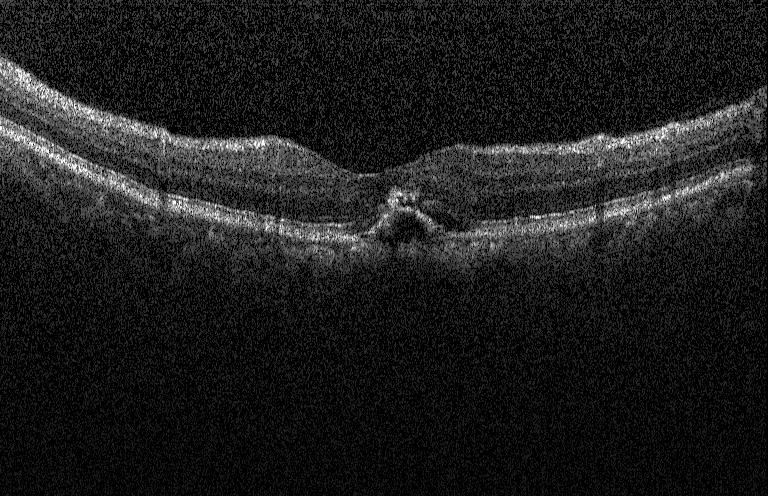
Choroidal neovascularization.